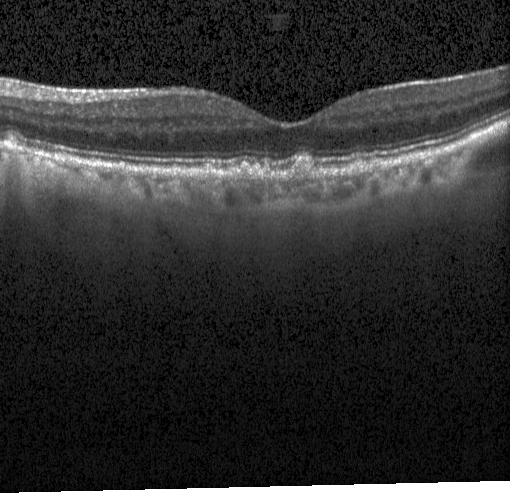

Centered on the fovea. Heidelberg Spectralis. Spectral-domain OCT. OCT line scan
Finding: multiple drusen.